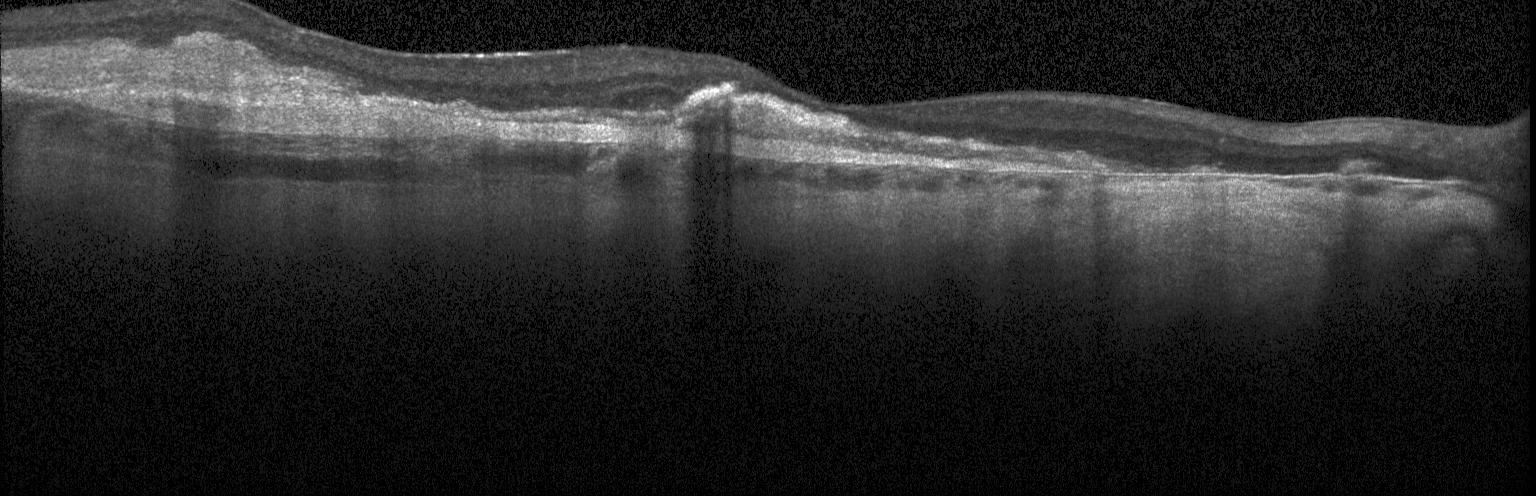
Retinal OCT cross-section; macular scan; spectral-domain optical coherence tomography. Diagnosis: choroidal neovascularization.